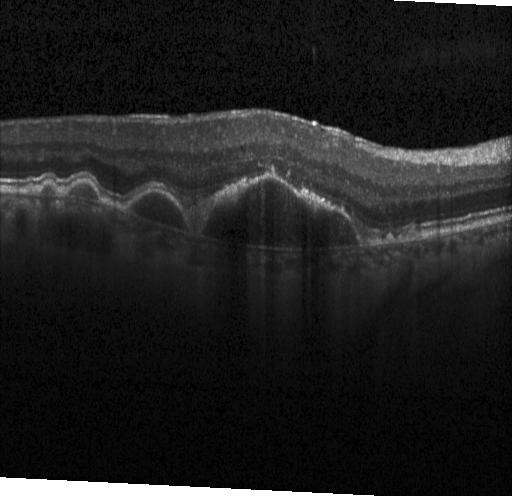
Spectral-domain optical coherence tomography. Heidelberg Spectralis. Horizontal scan through the fovea. OCT line scan — Impression: a choroidal neovascular membrane.